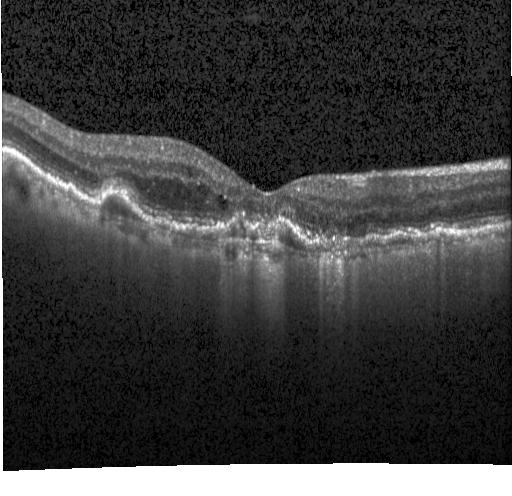
Horizontal scan through the fovea; Heidelberg Spectralis; optical coherence tomography scan; spectral-domain optical coherence tomography.
Macular OCT: choroidal neovascularization.